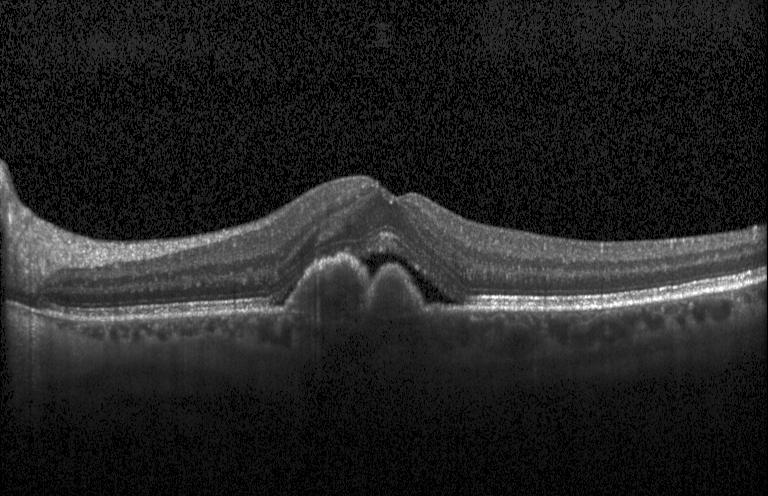 Optical coherence tomography scan, acquired on a Heidelberg Spectralis — Diagnosis: choroidal neovascularization.